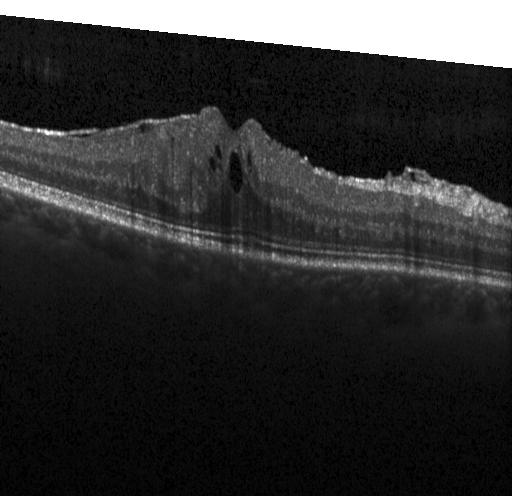

Through the macula. Optical coherence tomography B-scan. SD-OCT. Acquired on a Heidelberg Spectralis
Impression: diabetic macular edema (DME).